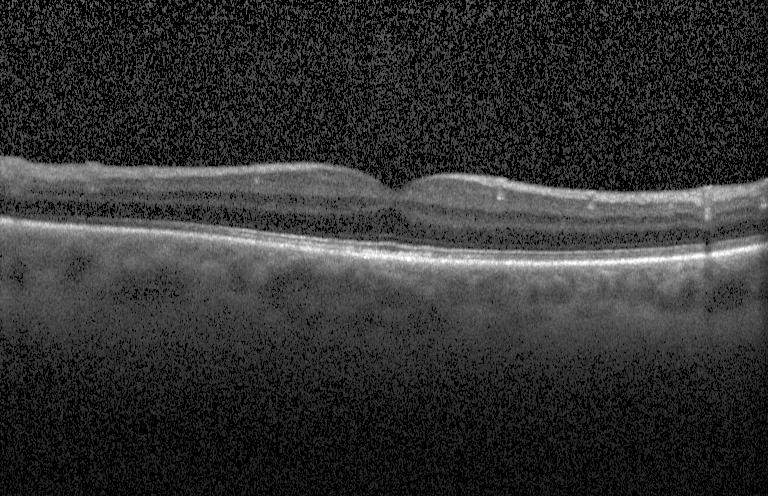 Centered on the fovea; OCT B-scan; Heidelberg Spectralis. Finding: no choroidal neovascularization, no diabetic macular edema, and no drusen.